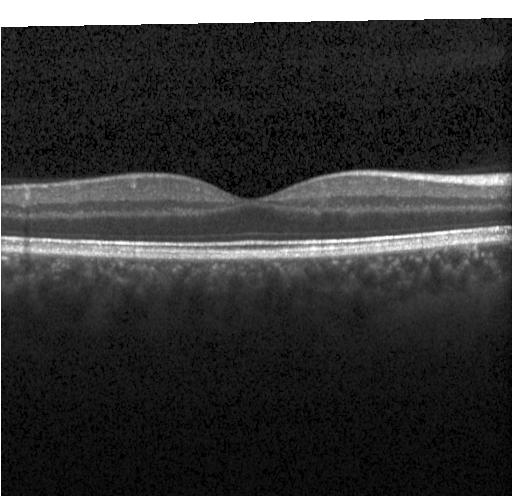
Diagnosis: no evidence of choroidal neovascularization, diabetic macular edema, or drusen.